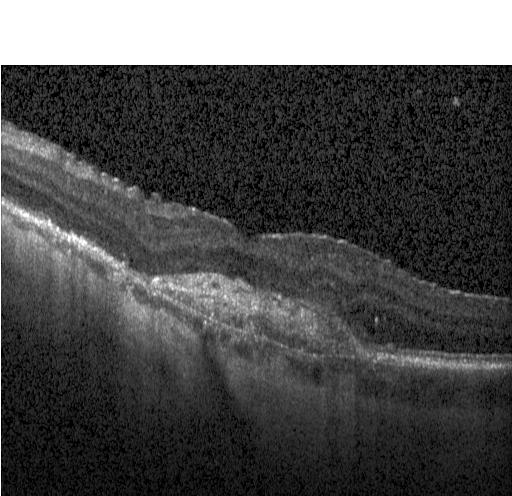 OCT finding: a choroidal neovascular membrane.